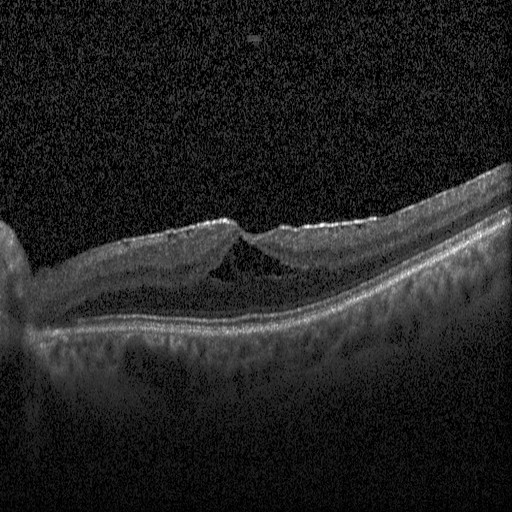

Diagnosis: DME.